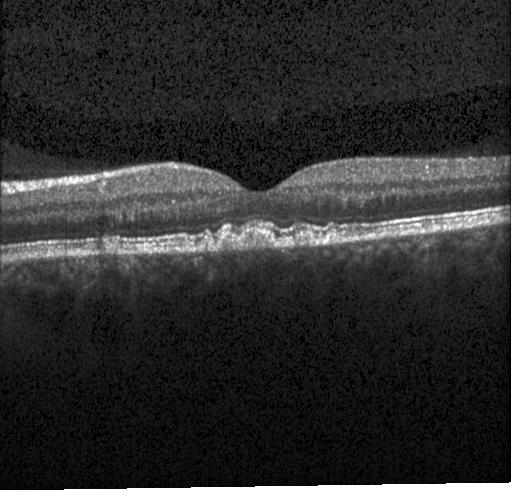 Acquired on a Heidelberg Spectralis; optical coherence tomography scan.
OCT finding: multiple drusen.